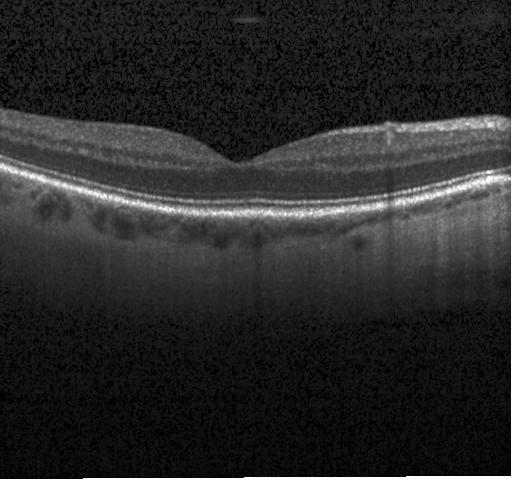 OCT B-scan, macular scan. Diagnosis: no choroidal neovascularization, diabetic macular edema, or drusen.